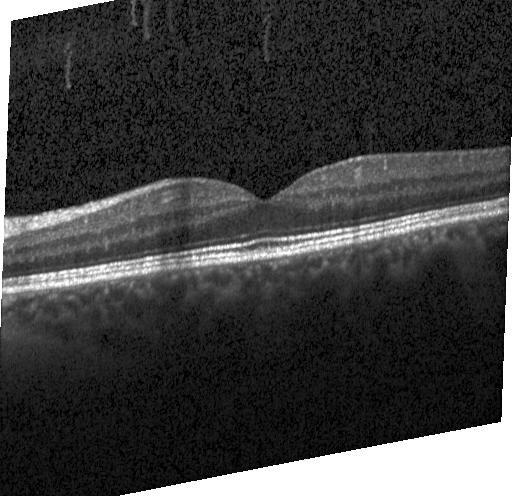 Optical coherence tomography scan — The scan shows no choroidal neovascularization, diabetic macular edema, or drusen.